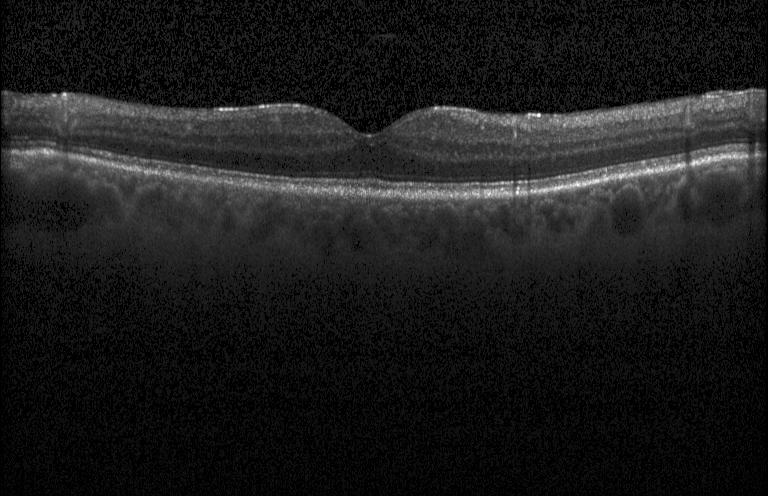 Horizontal scan through the fovea, instrument: Heidelberg Spectralis, OCT B-scan.
Impression: no evidence of CNV, DME, or drusen.